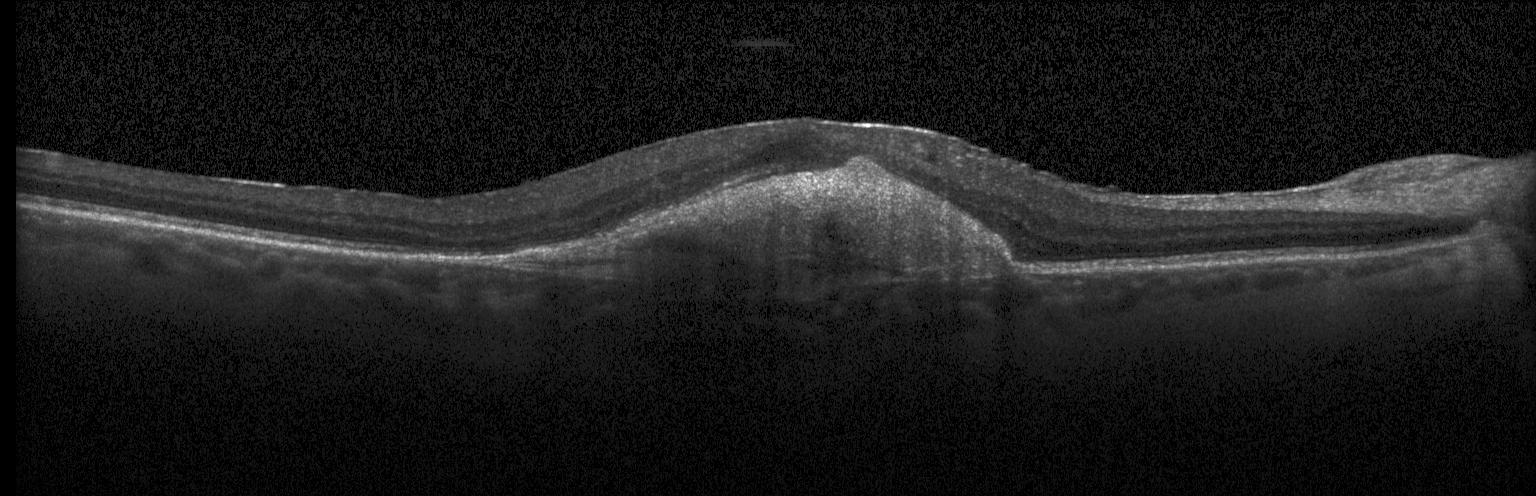

OCT finding: a choroidal neovascular membrane.